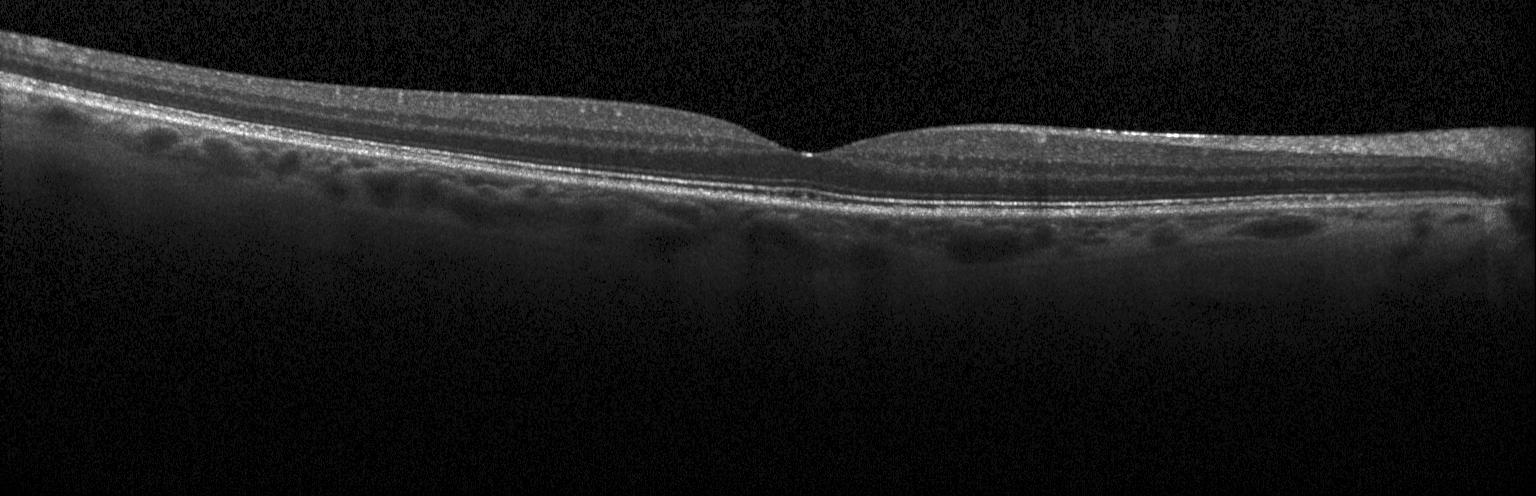

Retinal OCT B-scan
Finding: no choroidal neovascularization, diabetic macular edema, or drusen.